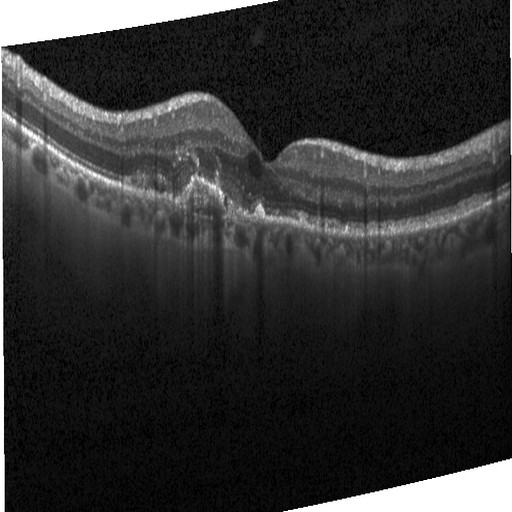

Retinal OCT cross-section showing diabetic macular edema (DME).